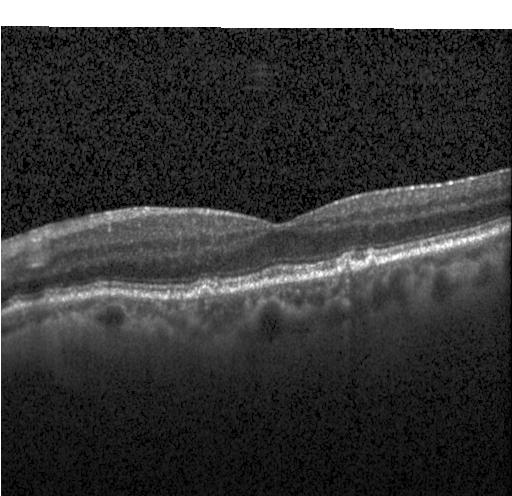 Finding: multiple drusen.